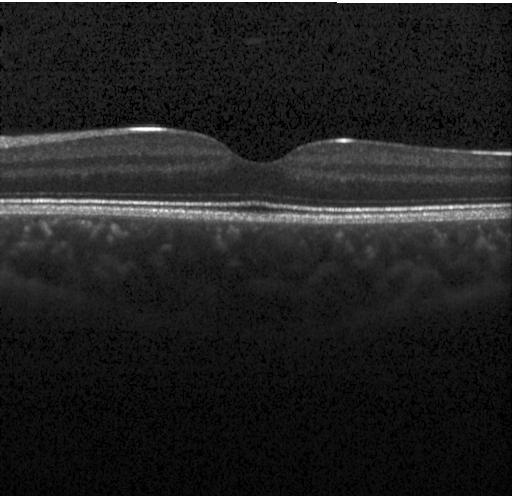
Horizontal scan through the fovea. Spectral-domain OCT. Retinal OCT cross-section. Instrument: Heidelberg Spectralis — OCT finding: no choroidal neovascularization, no diabetic macular edema, and no drusen.